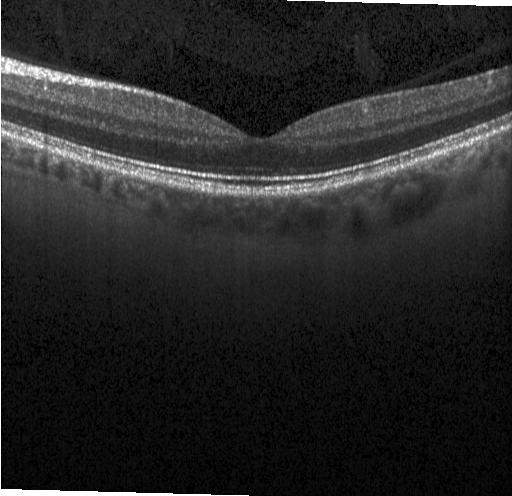
Macular OCT: no evidence of CNV, DME, or drusen.